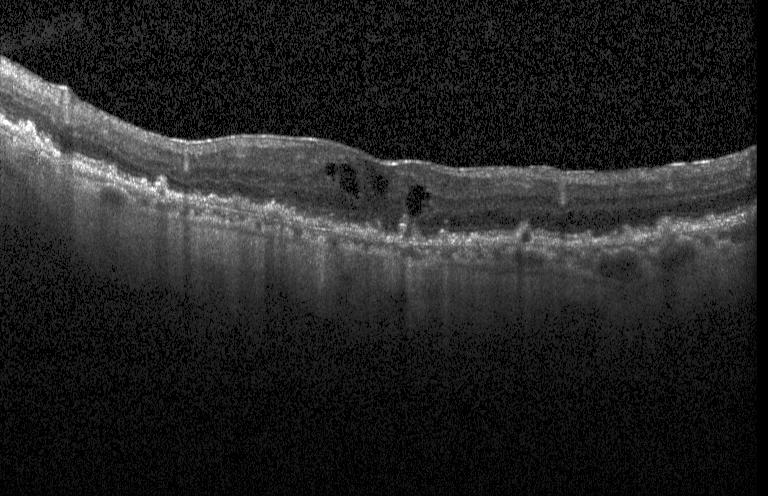 Optical coherence tomography scan
Diagnosis: a choroidal neovascular membrane.